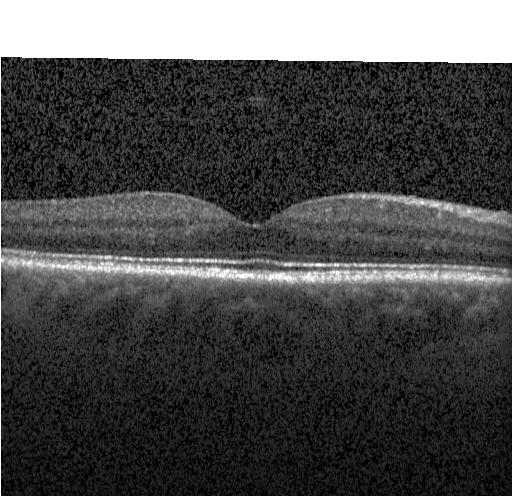
Finding: neither choroidal neovascularization, diabetic macular edema, nor drusen.